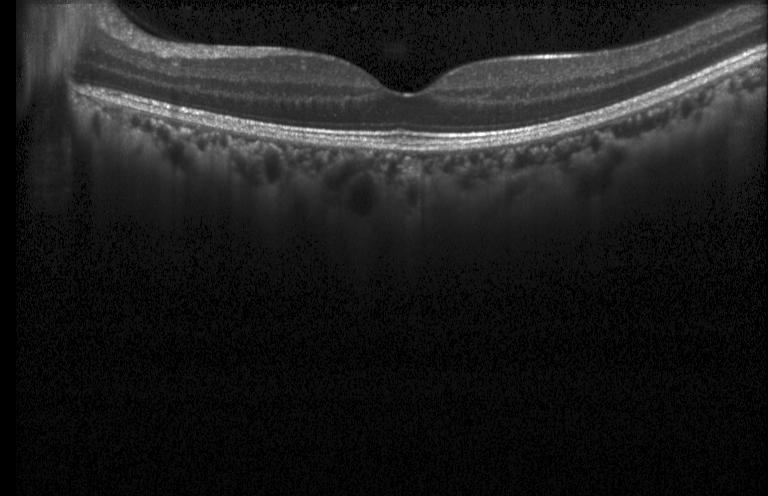 Diagnosis: neither CNV, DME, nor drusen.